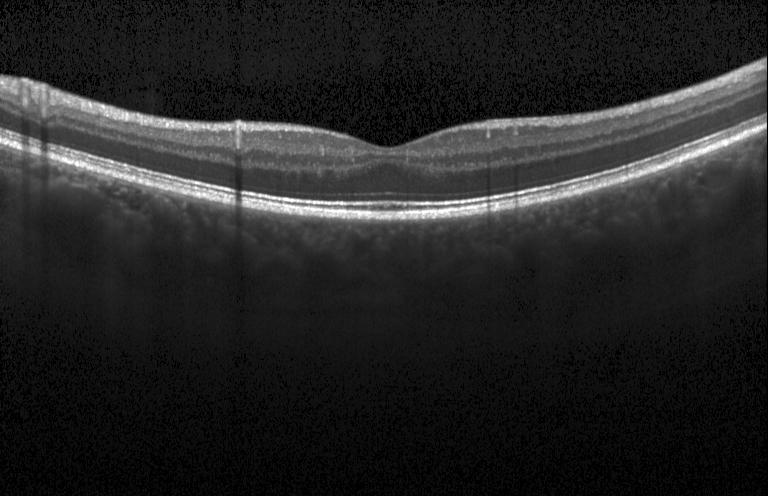

Heidelberg Spectralis. Retinal OCT B-scan
Diagnosis: neither CNV, DME, nor drusen.